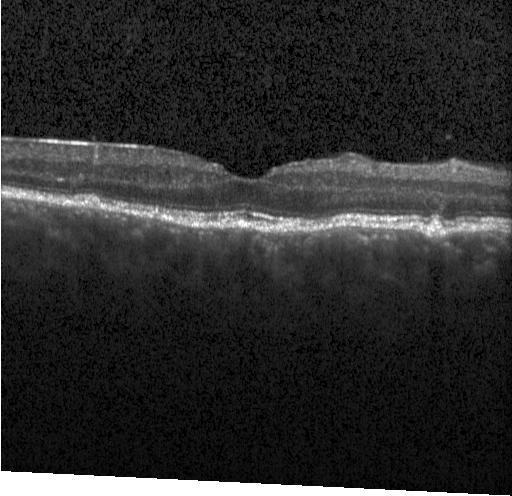 Spectral-domain optical coherence tomography · optical coherence tomography scan · macular scan · acquired on a Heidelberg Spectralis.
Diagnosis: no CNV, no DME, and no drusen.